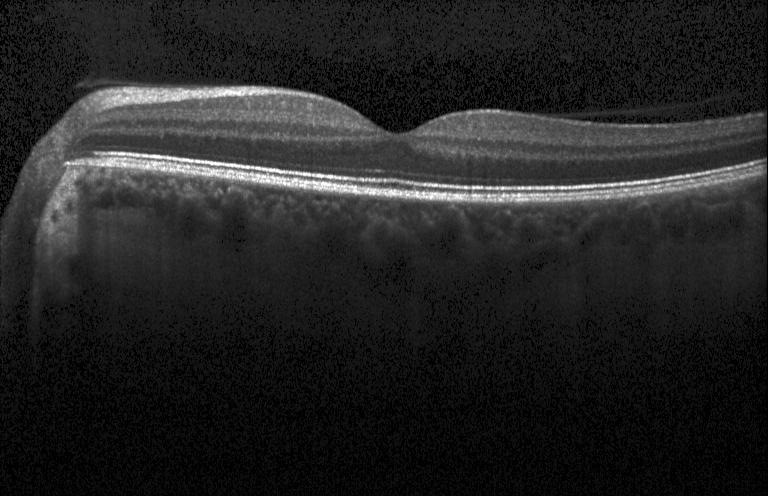
Spectral-domain OCT, through the macula, retinal OCT B-scan — Impression: neither choroidal neovascularization, diabetic macular edema, nor drusen.